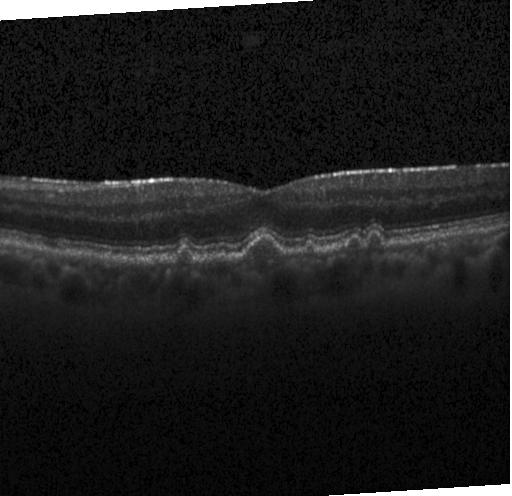 Assessment: sub-RPE drusenoid deposits.